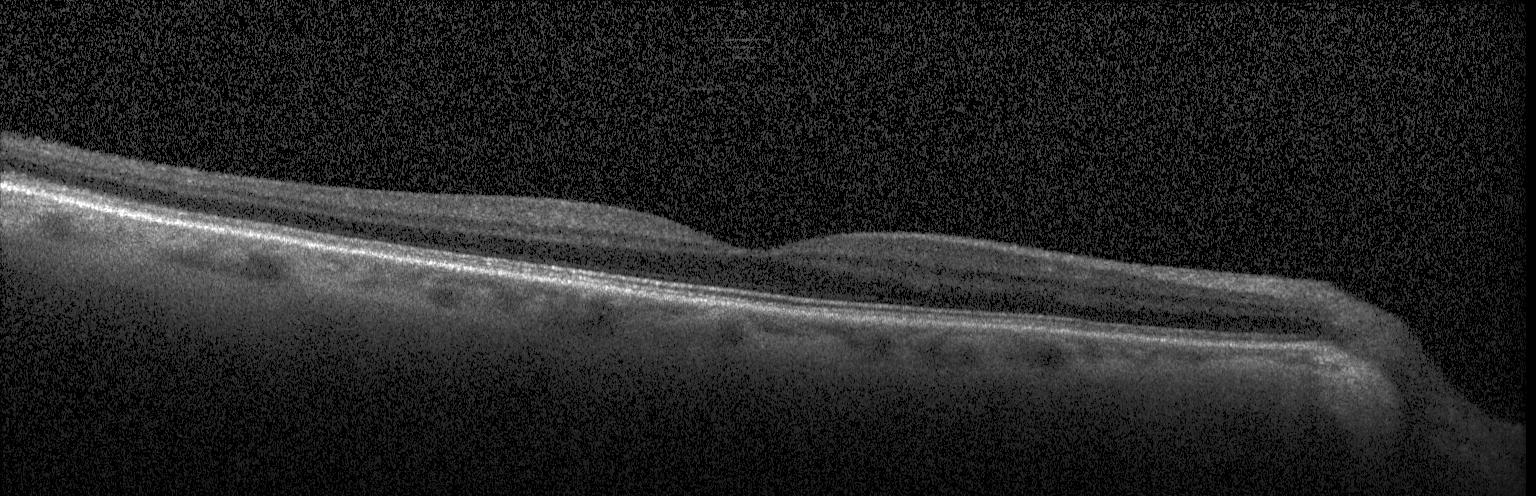

Optical coherence tomography B-scan.
Finding: neither CNV, DME, nor drusen.